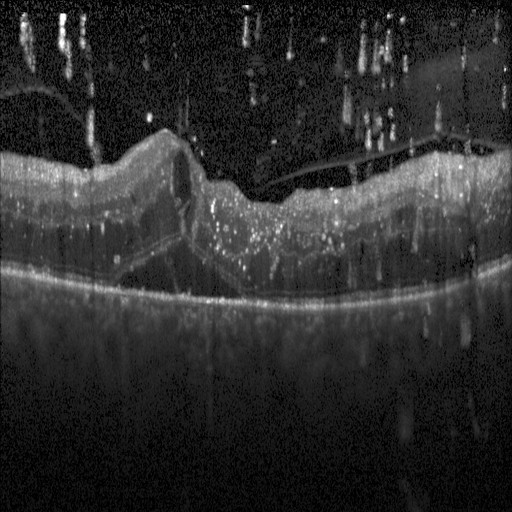

Diagnosis: DME.